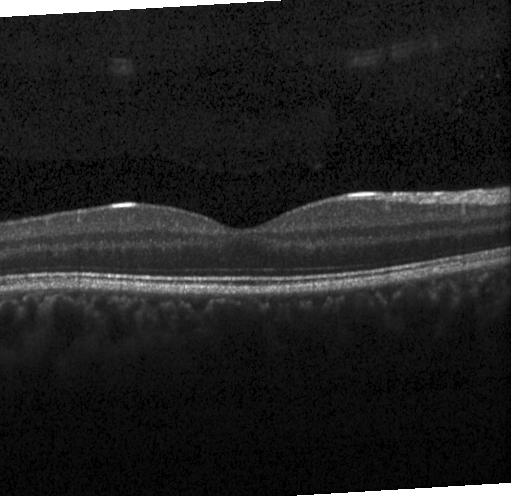
Macular scan, retinal OCT B-scan, instrument: Heidelberg Spectralis — This B-scan demonstrates neither choroidal neovascularization, diabetic macular edema, nor drusen.